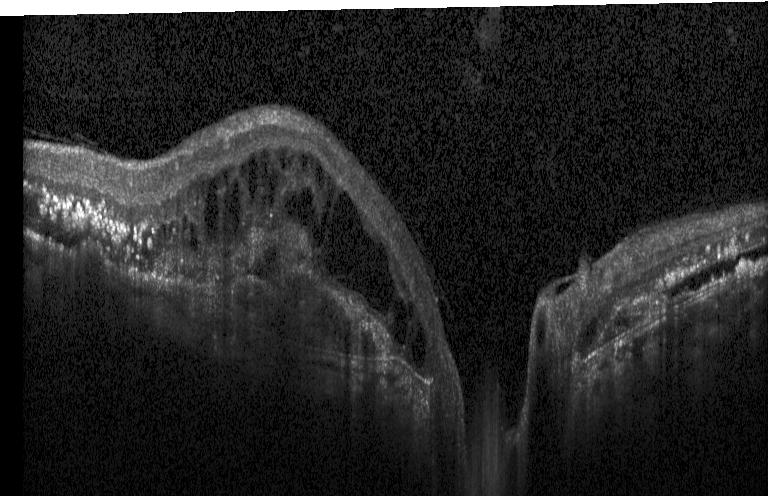 Macular OCT demonstrating a choroidal neovascular membrane.